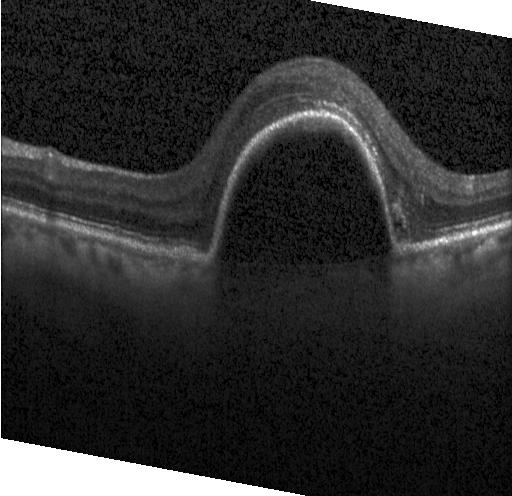 OCT B-scan · fovea-centered
Dx: CNV.